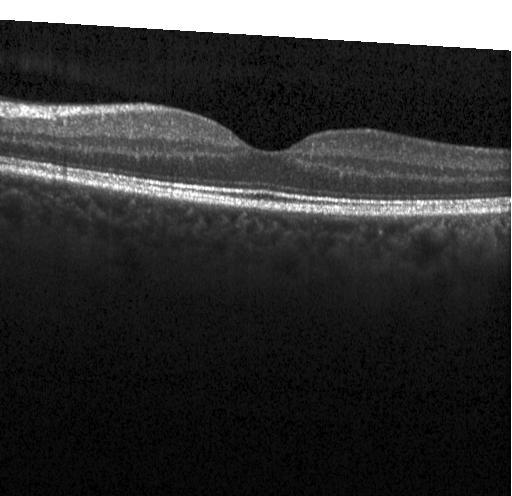
Assessment: no choroidal neovascularization, no diabetic macular edema, and no drusen.